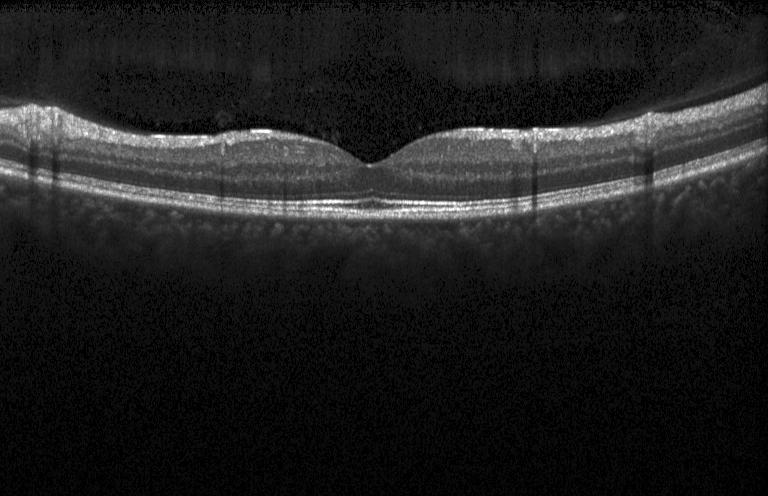 OCT line scan; horizontal scan through the fovea; SD-OCT — Diagnosis: no choroidal neovascularization, diabetic macular edema, or drusen.